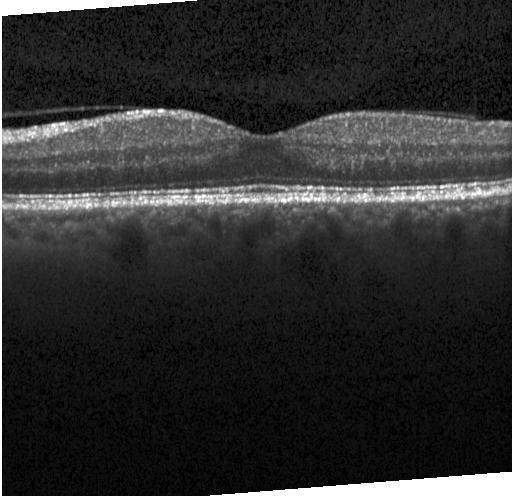

Optical coherence tomography B-scan. Centered on the fovea. Instrument: Heidelberg Spectralis. Spectral-domain optical coherence tomography — This B-scan demonstrates no CNV, DME, or drusen.